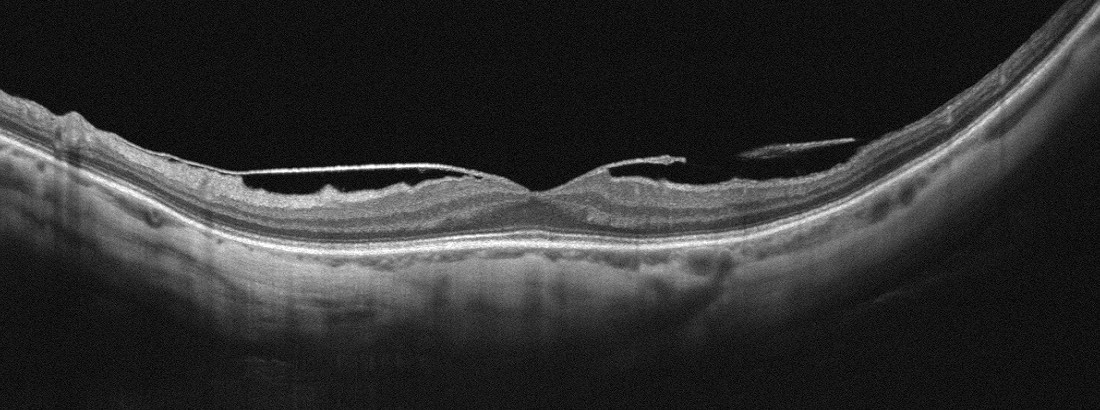

OCT scan showing epiretinal membrane.